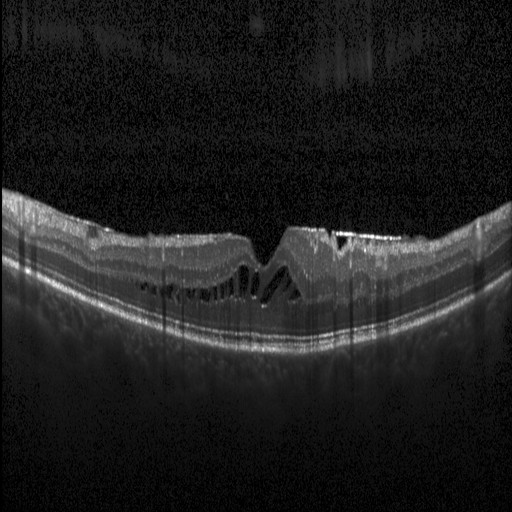
Spectral-domain OCT B-scan: diabetic macular edema.